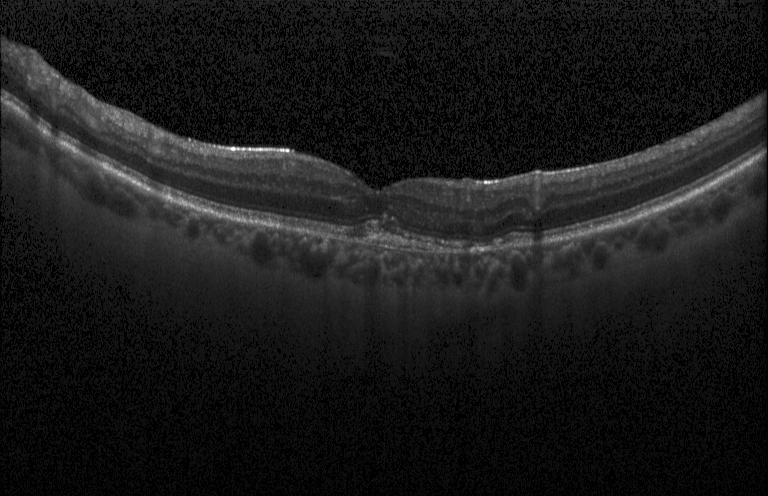 SD-OCT · OCT line scan · instrument: Heidelberg Spectralis
Finding: CNV.